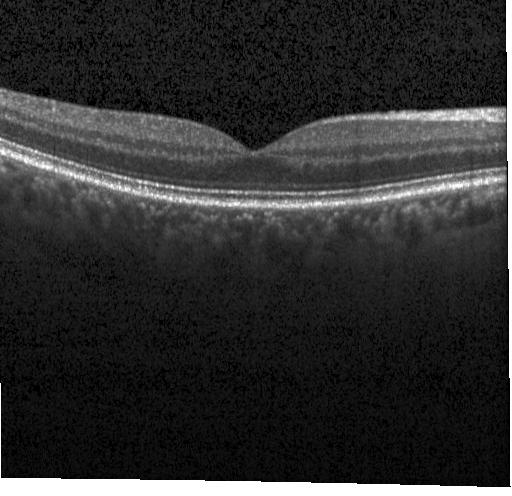

Centered on the fovea; spectral-domain optical coherence tomography; OCT B-scan — Diagnosis: no evidence of choroidal neovascularization, diabetic macular edema, or drusen.